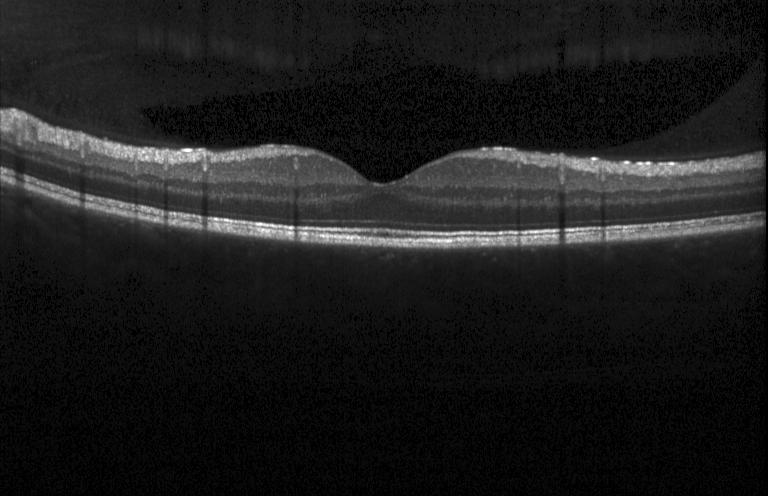
OCT B-scan.
The scan shows no CNV, DME, or drusen.